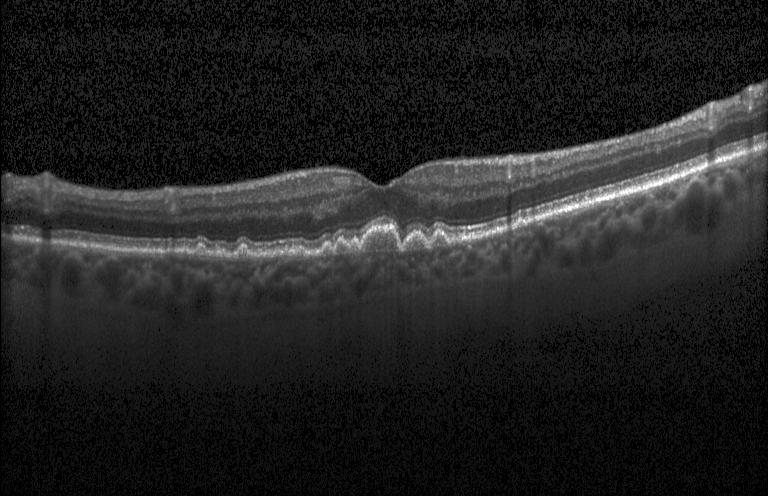 OCT line scan
Diagnosis: multiple drusen.